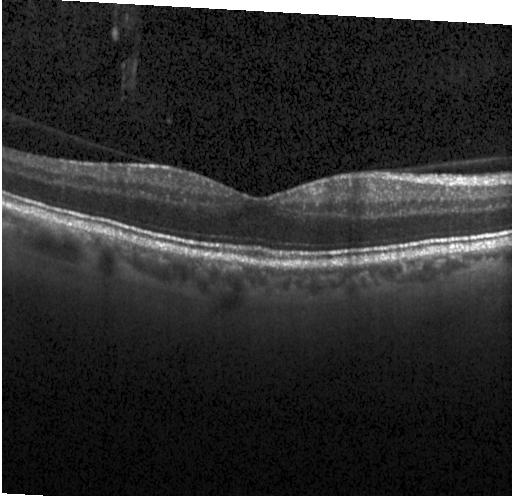 Fovea-centered · spectral-domain OCT · retinal OCT B-scan
Diagnosis: no choroidal neovascularization, no diabetic macular edema, and no drusen.